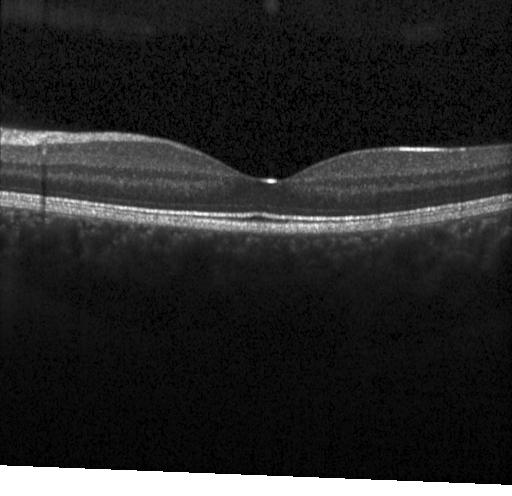
Optical coherence tomography B-scan — Assessment: no choroidal neovascularization, no diabetic macular edema, and no drusen.